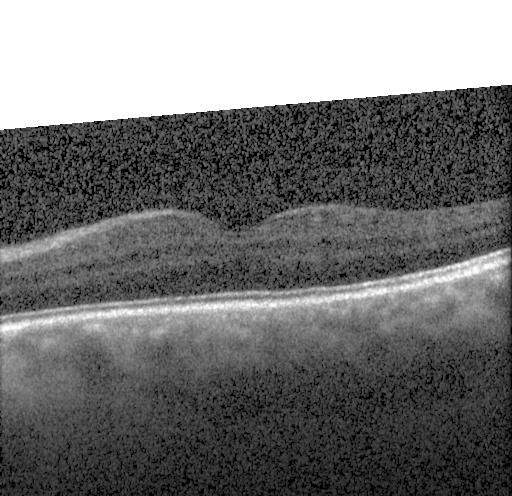

No choroidal neovascularization, no diabetic macular edema, and no drusen.